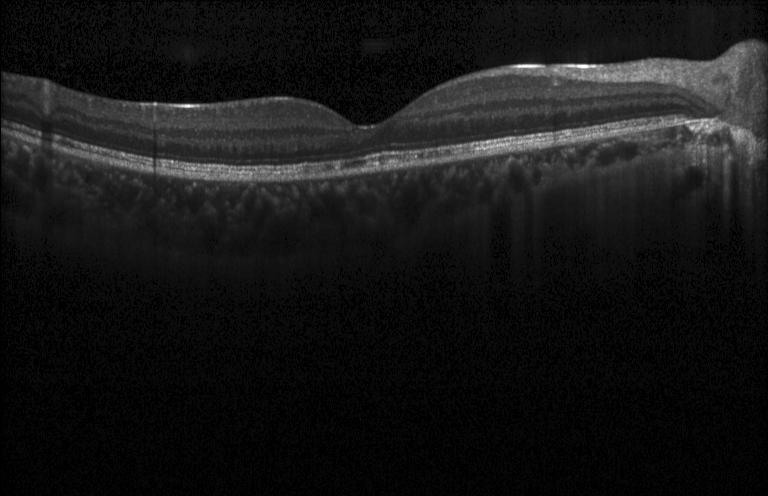
Instrument: Heidelberg Spectralis. SD-OCT. Horizontal scan through the fovea. Retinal OCT cross-section. Macular OCT: neither choroidal neovascularization, diabetic macular edema, nor drusen.